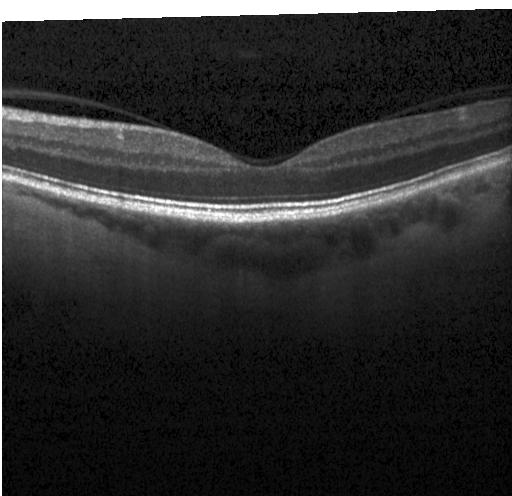 Macular OCT demonstrating no choroidal neovascularization, no diabetic macular edema, and no drusen.